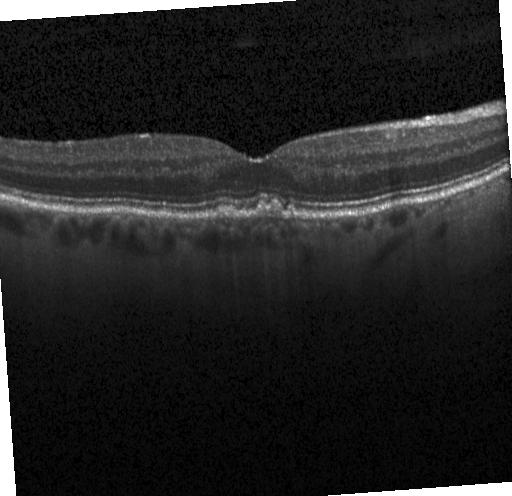

Spectral-domain OCT B-scan: drusen.